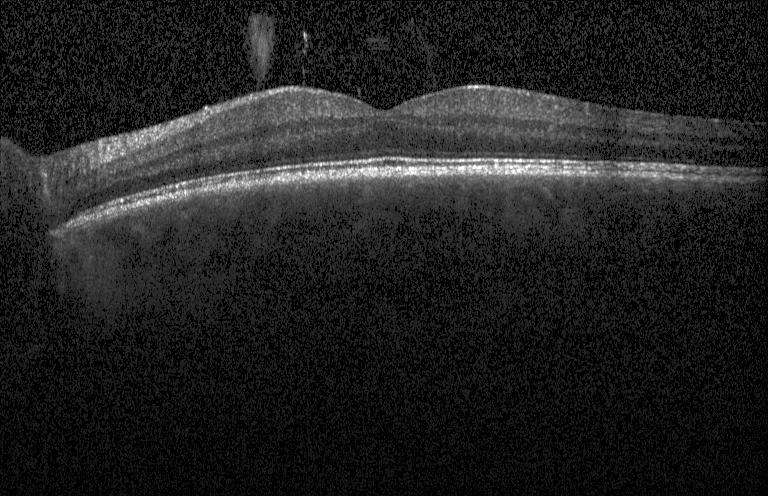
Diagnosis: no evidence of choroidal neovascularization, diabetic macular edema, or drusen.